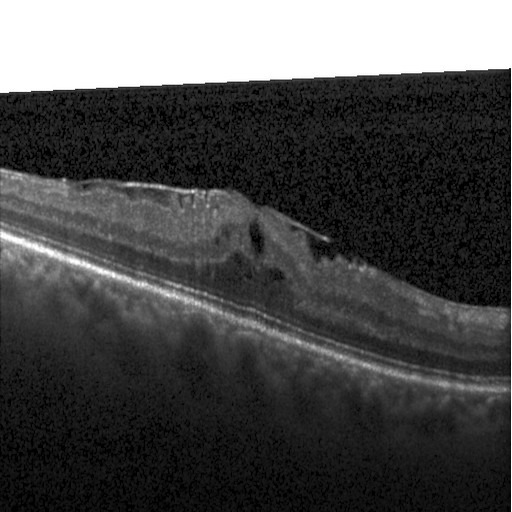

Spectral-domain optical coherence tomography · OCT line scan · through the macula · acquired on a Heidelberg Spectralis — DME.